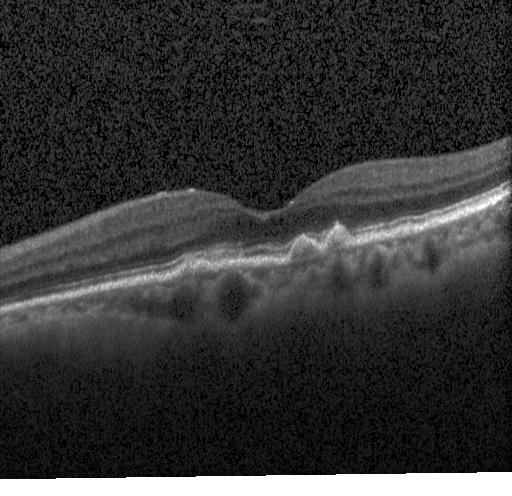
Finding: multiple drusen.